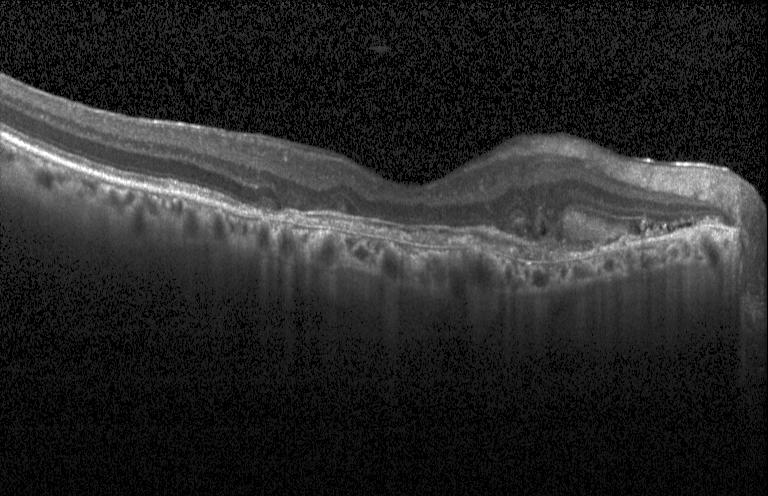
OCT line scan · macular scan
Impression: choroidal neovascularization (CNV).